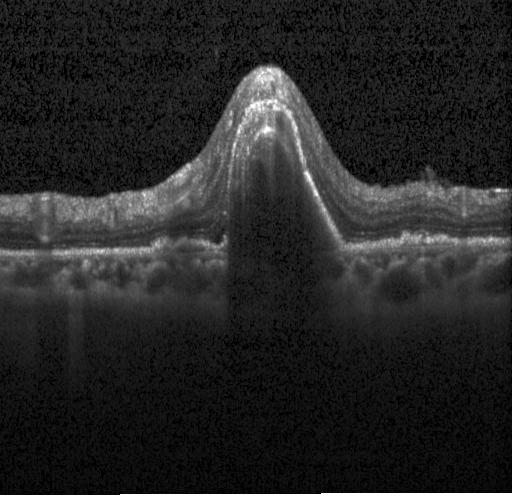

Retinal OCT cross-section · spectral-domain OCT. The scan shows a choroidal neovascular membrane.